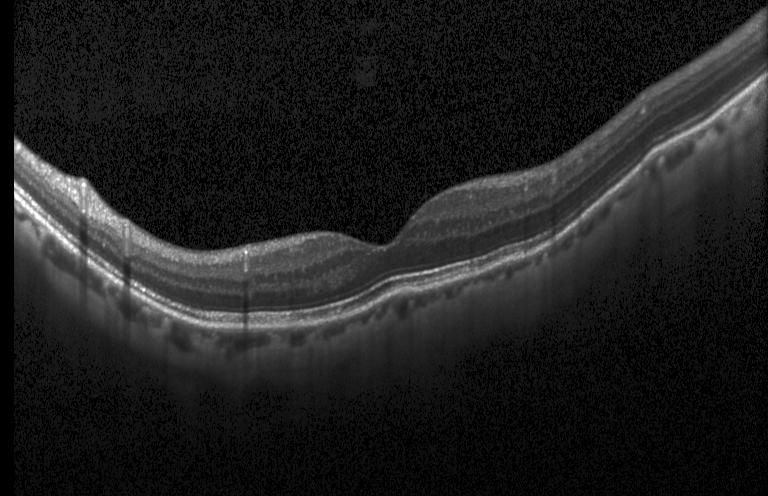 SD-OCT; OCT line scan; instrument: Heidelberg Spectralis.
Diagnosis: neither choroidal neovascularization, diabetic macular edema, nor drusen.